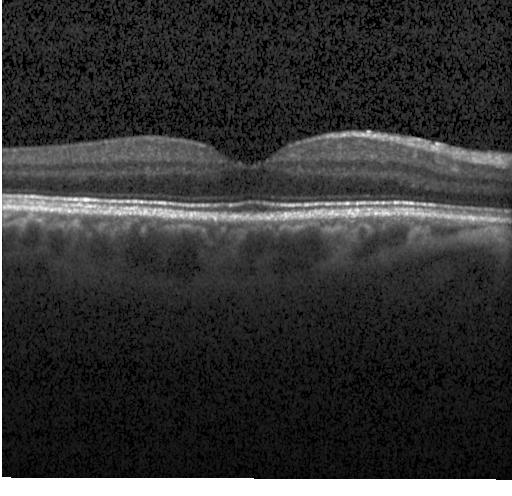
Diagnosis: neither choroidal neovascularization, diabetic macular edema, nor drusen.